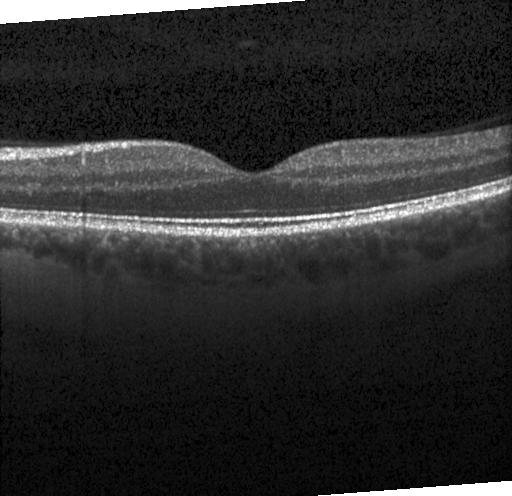
Impression: no evidence of CNV, DME, or drusen.